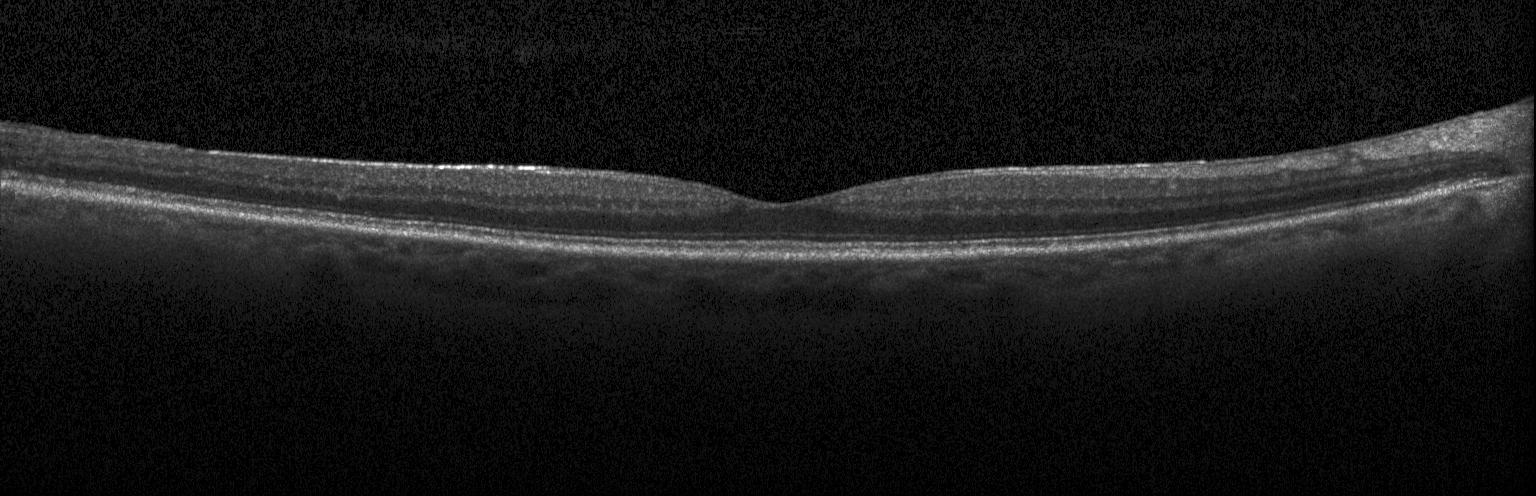
Through the macula; spectral-domain optical coherence tomography; retinal OCT cross-section; Heidelberg Spectralis. This B-scan demonstrates neither CNV, DME, nor drusen.